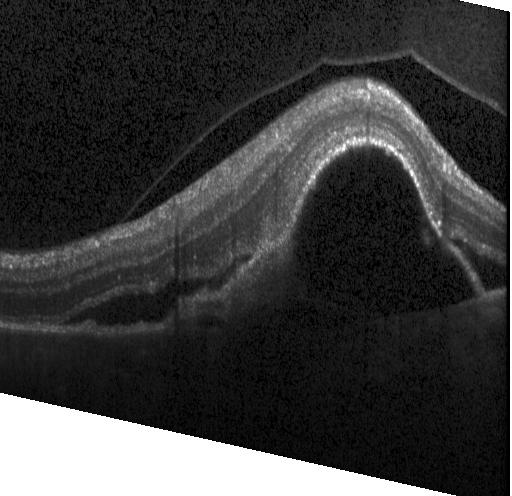

Optical coherence tomography scan.
Diagnosis: a choroidal neovascular membrane.